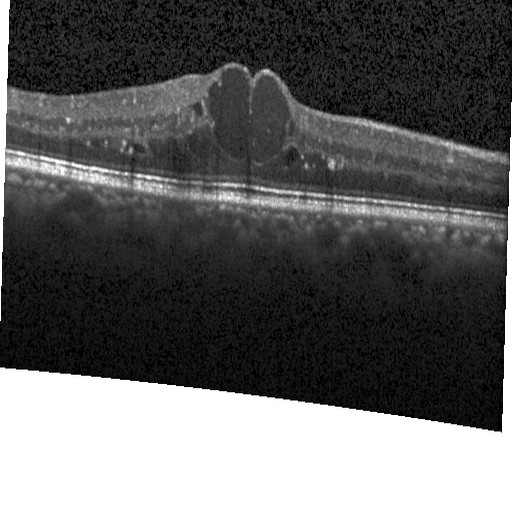
OCT finding: diabetic macular edema (DME).